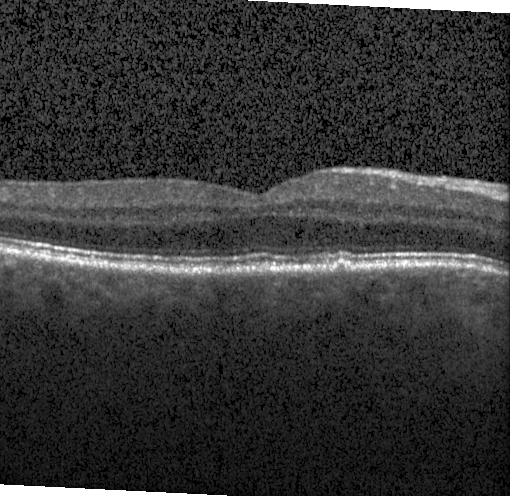

Macular OCT: multiple drusen.